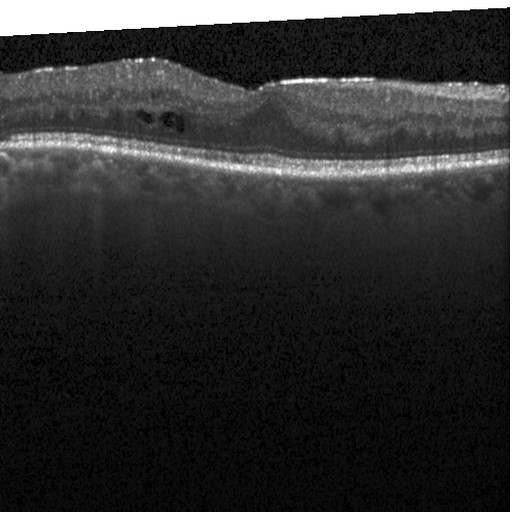 Macular OCT demonstrating DME.